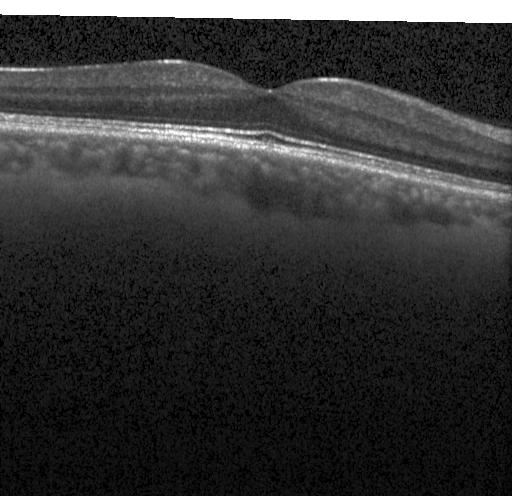
OCT B-scan. Macular OCT: no choroidal neovascularization, no diabetic macular edema, and no drusen.